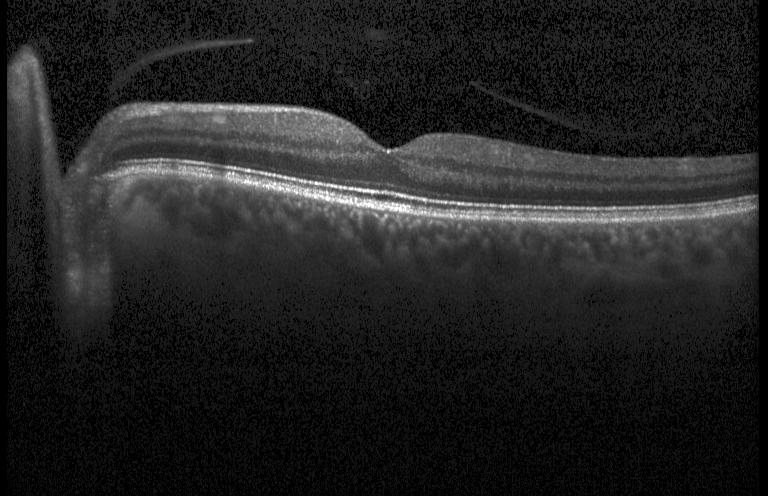 Spectral-domain OCT; optical coherence tomography B-scan; fovea-centered; Heidelberg Spectralis OCT system.
Finding: no choroidal neovascularization, no diabetic macular edema, and no drusen.